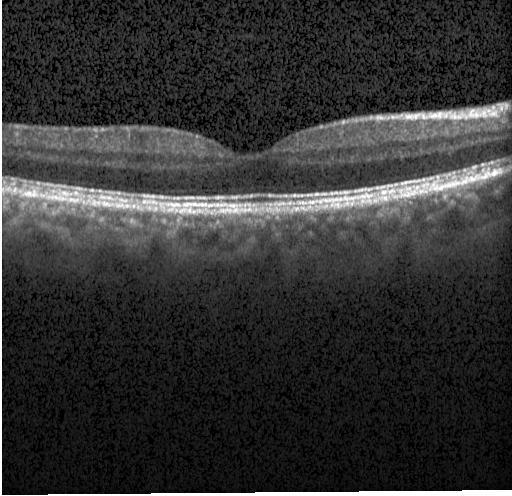 OCT finding: neither CNV, DME, nor drusen.